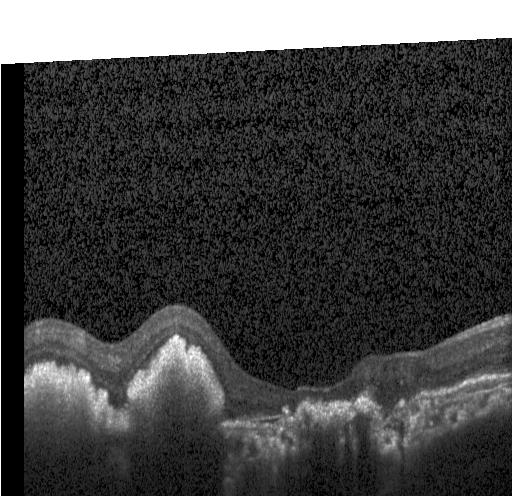
Macular OCT demonstrating choroidal neovascularization.